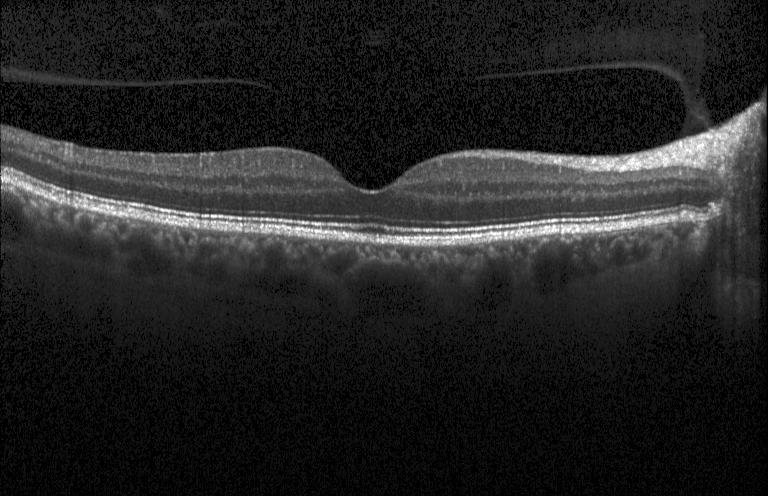
Instrument: Heidelberg Spectralis; optical coherence tomography scan; horizontal scan through the fovea — Finding: no evidence of CNV, DME, or drusen.